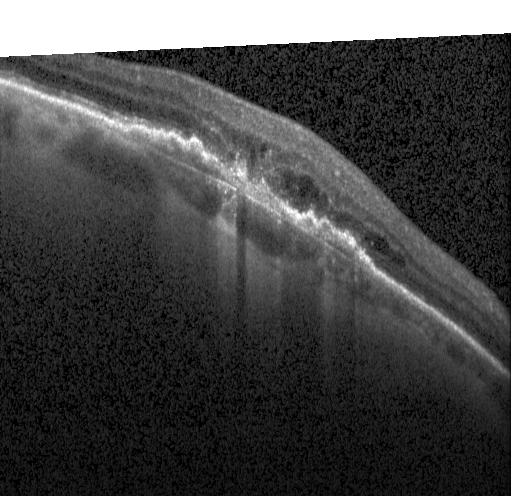
Finding: a choroidal neovascular membrane.